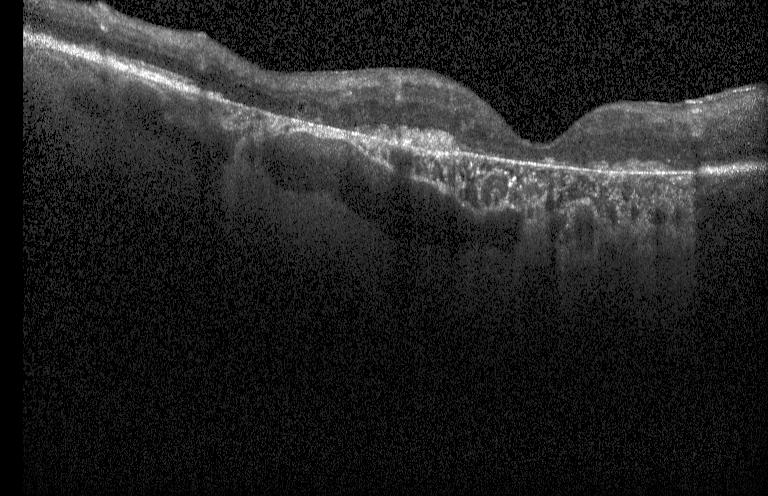 OCT B-scan showing a choroidal neovascular membrane.